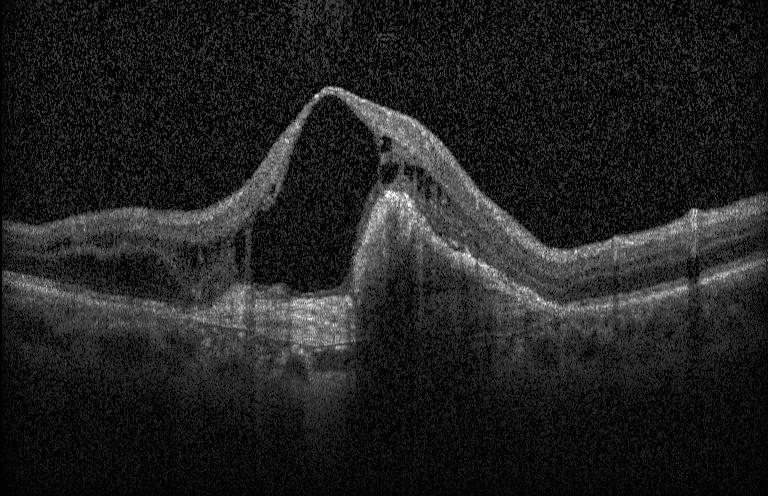

OCT B-scan. The scan shows choroidal neovascularization (CNV).